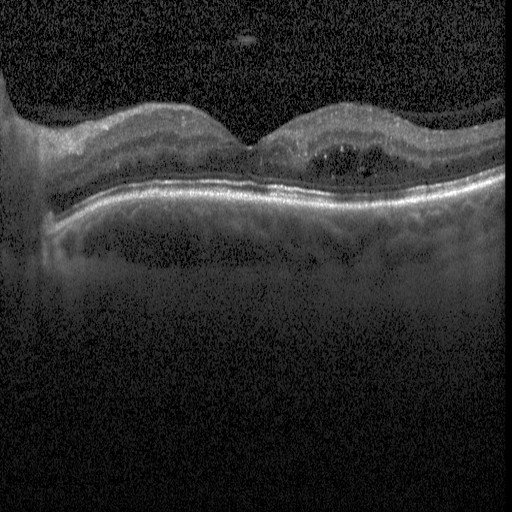 Retinal OCT B-scan · spectral-domain optical coherence tomography · Heidelberg Spectralis · centered on the fovea.
This B-scan demonstrates diabetic macular edema (DME).